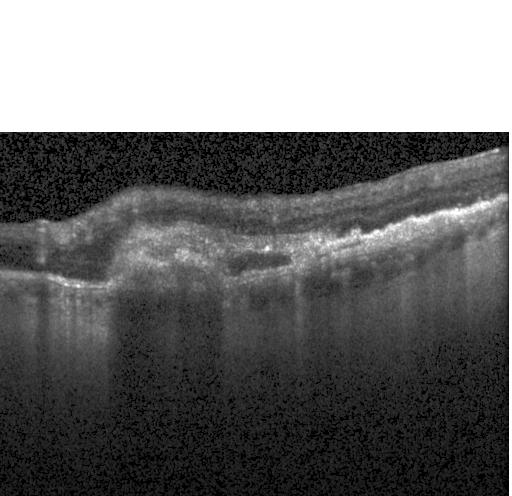
Macular OCT: choroidal neovascularization.